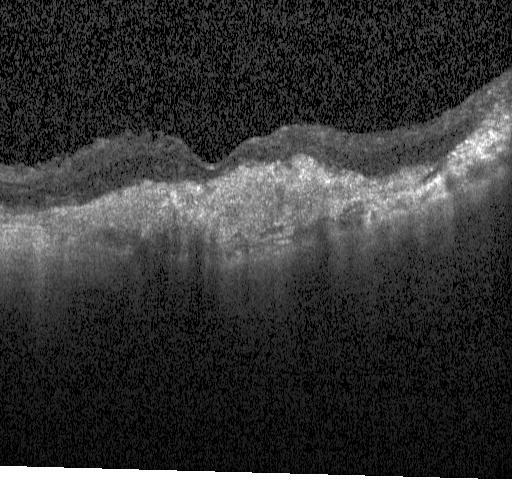

Heidelberg Spectralis; retinal OCT cross-section; spectral-domain optical coherence tomography; horizontal scan through the fovea — Impression: a choroidal neovascular membrane.